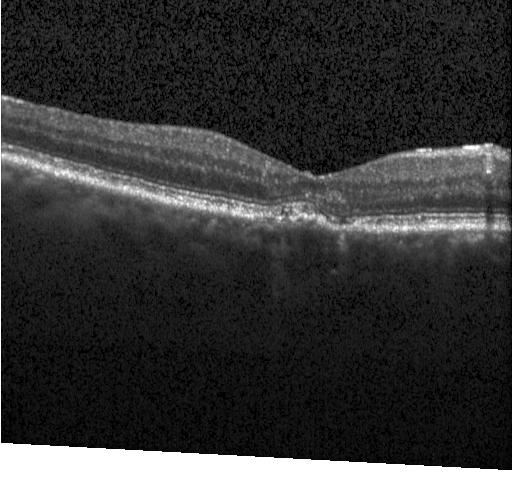
Retinal OCT cross-section showing sub-RPE drusenoid deposits.